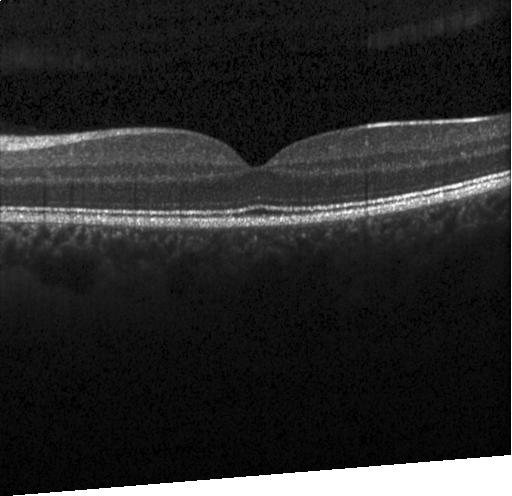

Acquired on a Heidelberg Spectralis · SD-OCT · horizontal scan through the fovea · retinal OCT cross-section — Impression: no CNV, no DME, and no drusen.